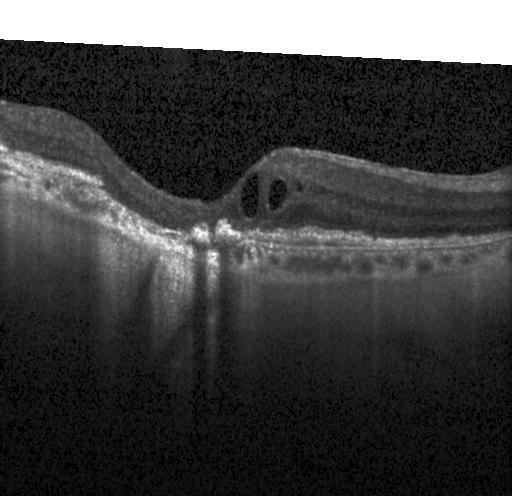
Retinal OCT B-scan.
Impression: CNV.